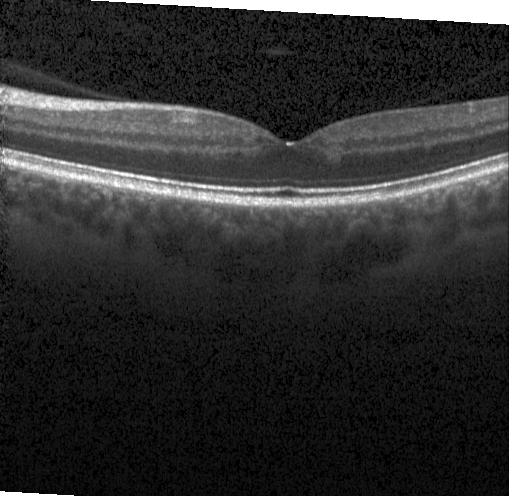

Impression: no choroidal neovascularization, diabetic macular edema, or drusen.